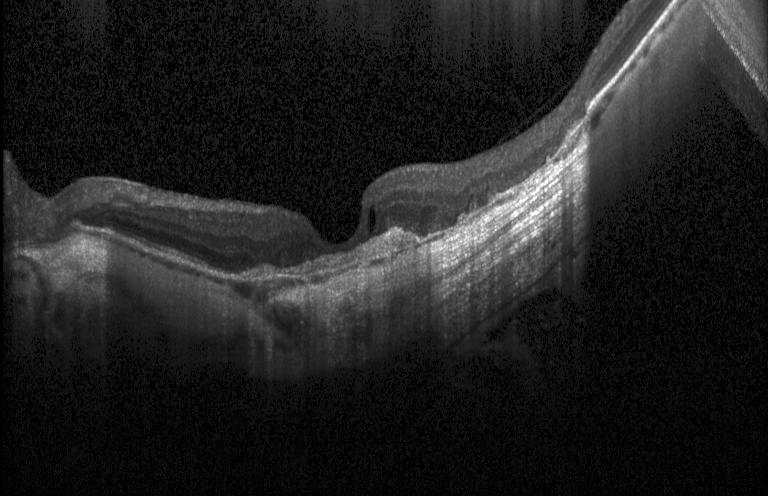
Heidelberg Spectralis. OCT line scan. Through the macula. Spectral-domain OCT. Dx: a choroidal neovascular membrane.